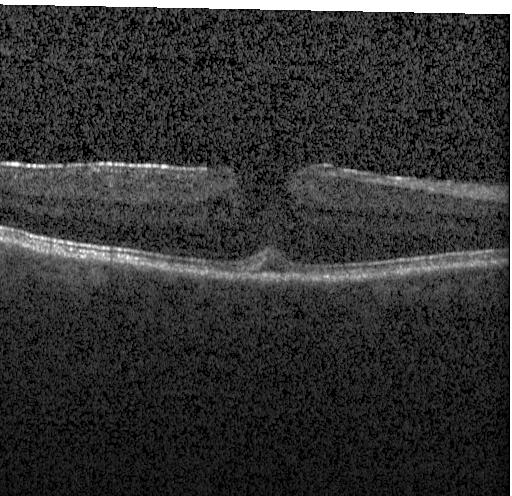 Dx: DME.